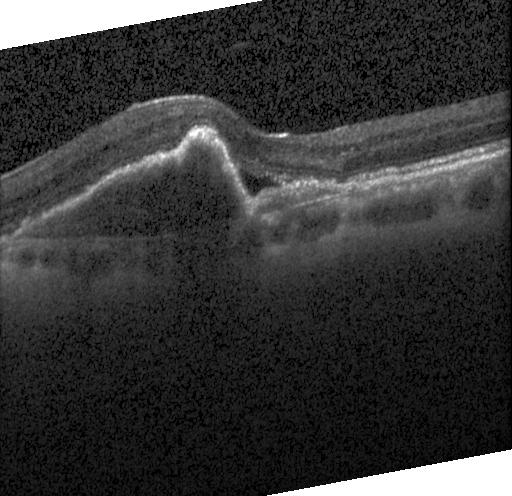

This B-scan demonstrates CNV.